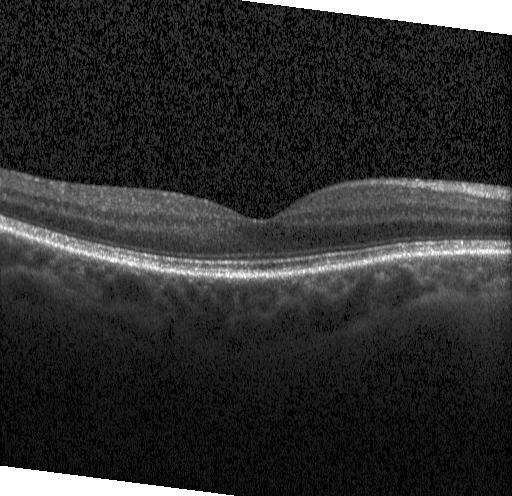
Retinal OCT B-scan · Heidelberg Spectralis. No choroidal neovascularization, diabetic macular edema, or drusen.